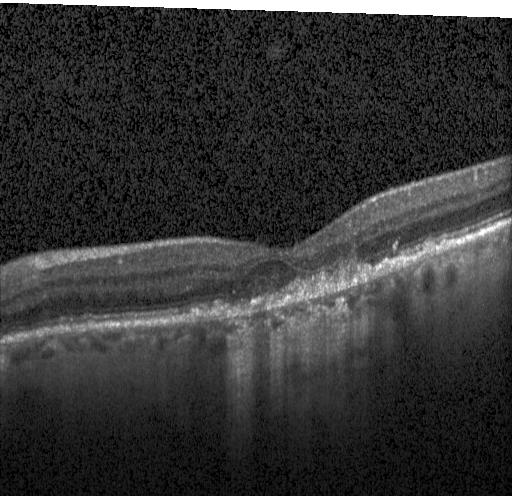

Macular scan · Heidelberg Spectralis OCT system · optical coherence tomography B-scan — Diagnosis: a choroidal neovascular membrane.